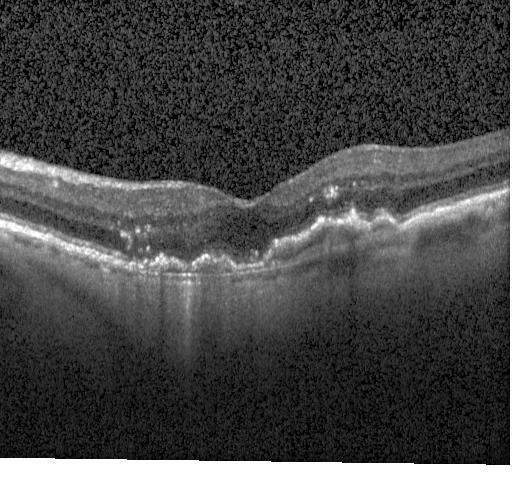
Retinal OCT B-scan · acquired on a Heidelberg Spectralis · through the macula. Diagnosis: CNV.